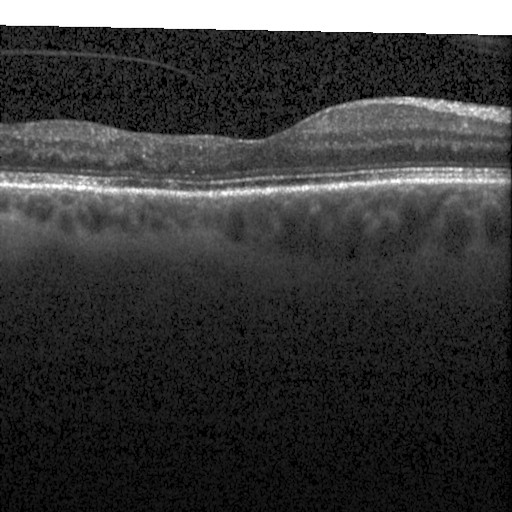
Impression: DME.